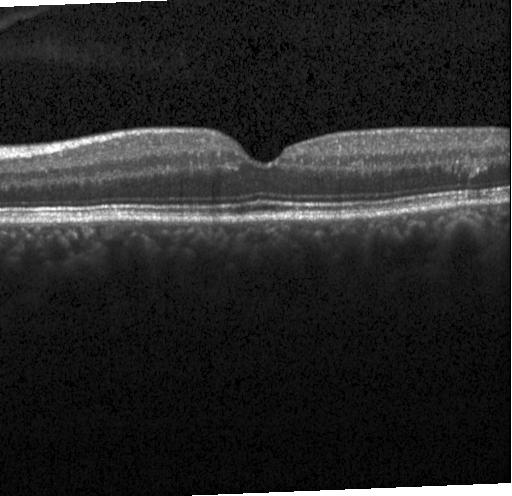
Fovea-centered, OCT line scan — Finding: neither CNV, DME, nor drusen.